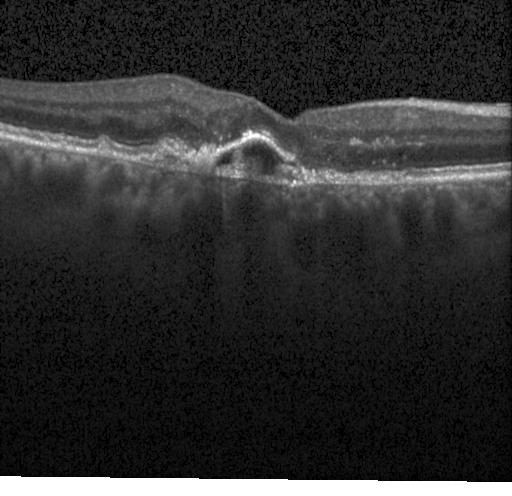 Heidelberg Spectralis, optical coherence tomography scan, macular scan, spectral-domain OCT. OCT finding: choroidal neovascularization.